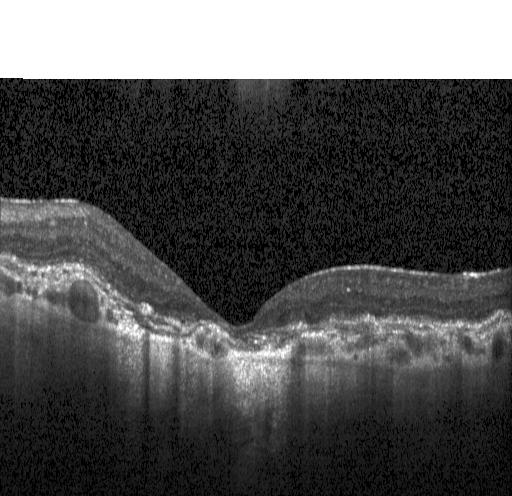
Optical coherence tomography scan; spectral-domain OCT
This B-scan demonstrates a choroidal neovascular membrane.